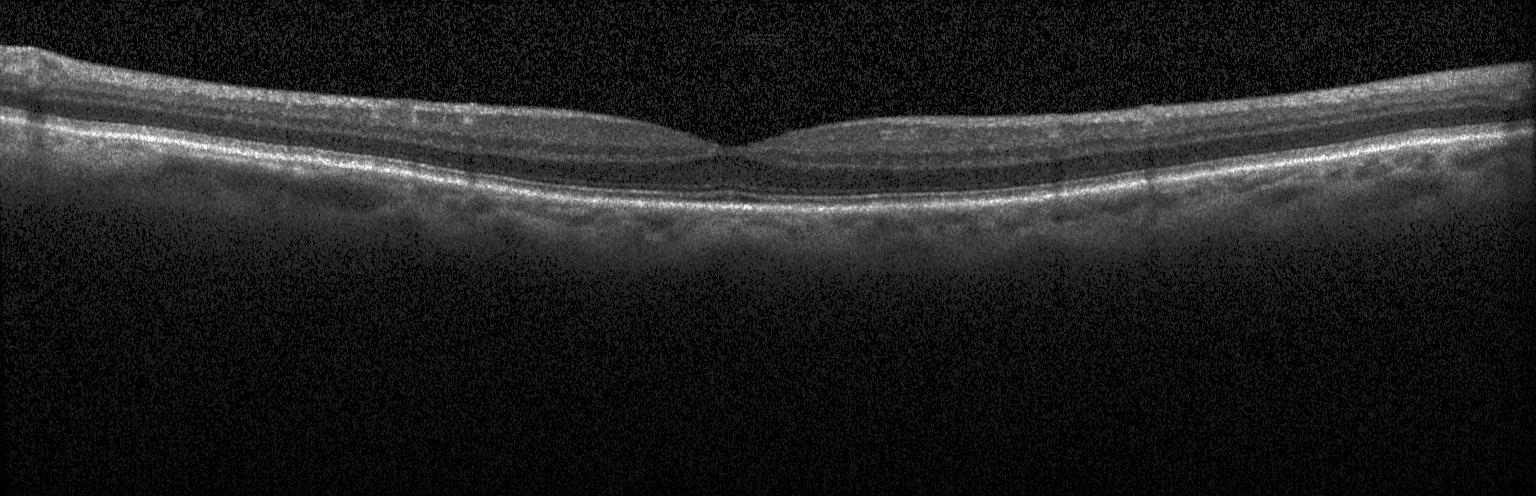 Spectral-domain OCT B-scan: no evidence of choroidal neovascularization, diabetic macular edema, or drusen.